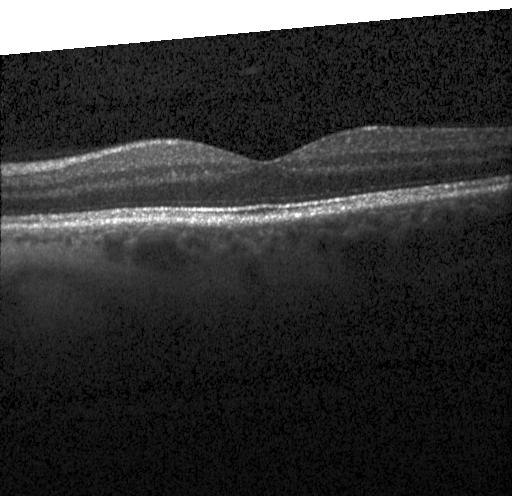

Optical coherence tomography scan
Finding: no evidence of choroidal neovascularization, diabetic macular edema, or drusen.